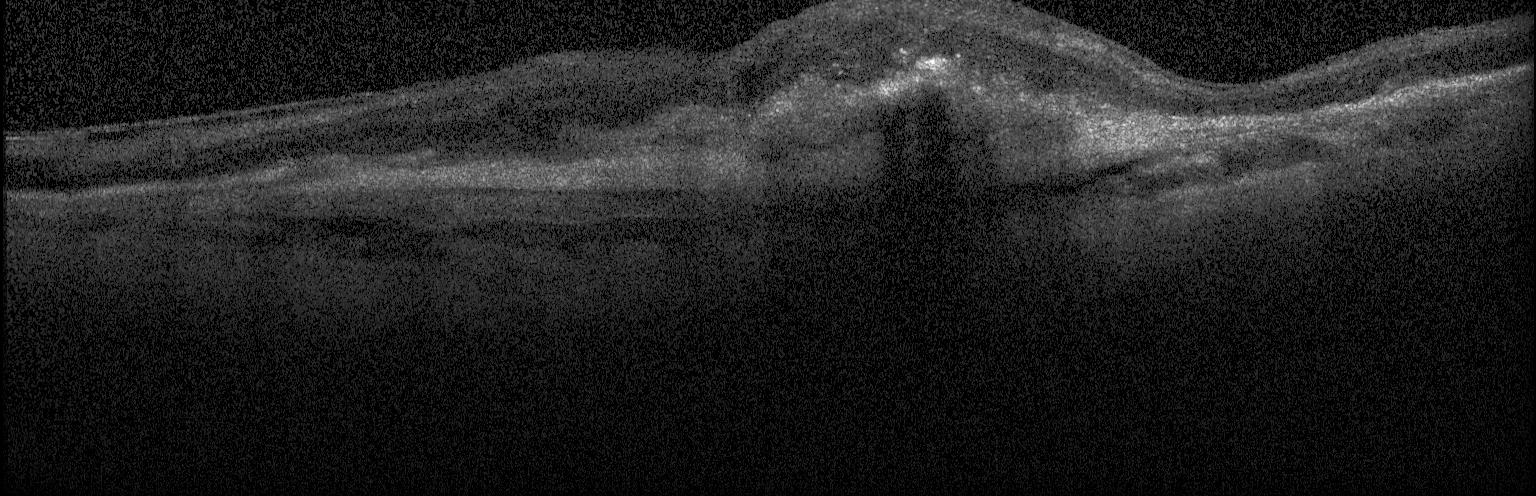 Acquired on a Heidelberg Spectralis · retinal OCT cross-section · fovea-centered.
Diagnosis: a choroidal neovascular membrane.